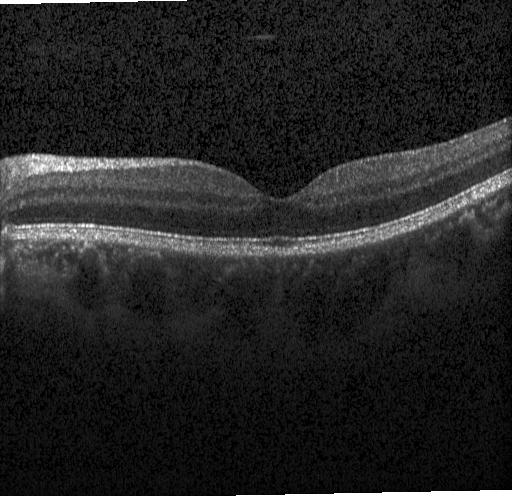
Diagnosis: no evidence of choroidal neovascularization, diabetic macular edema, or drusen.